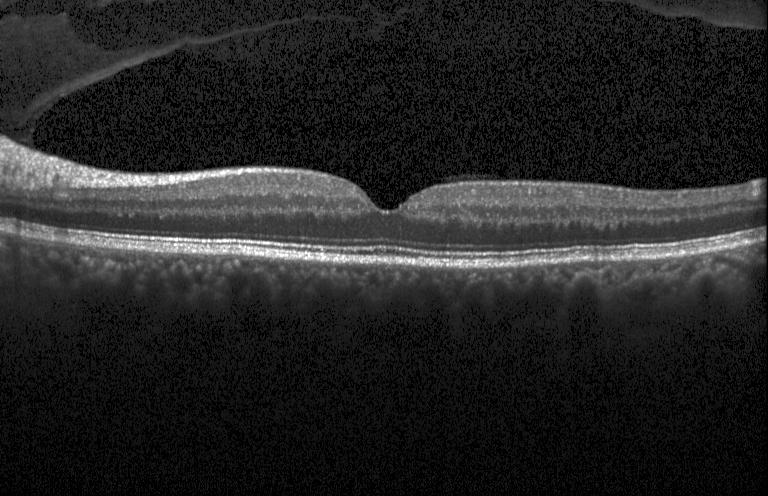

OCT B-scan. Through the macula. Heidelberg Spectralis OCT system. SD-OCT
OCT finding: neither choroidal neovascularization, diabetic macular edema, nor drusen.